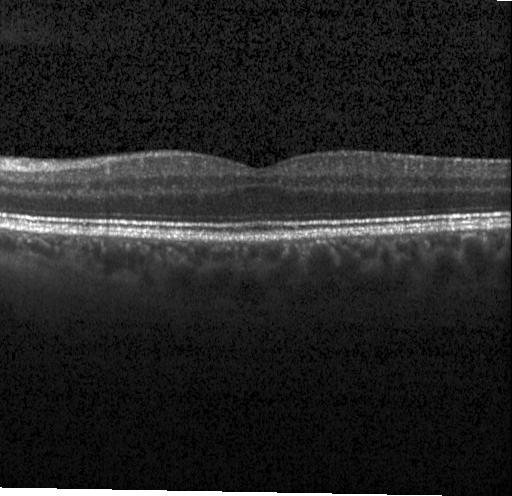
Horizontal scan through the fovea · SD-OCT · optical coherence tomography scan · Heidelberg Spectralis OCT system. Impression: no CNV, DME, or drusen.